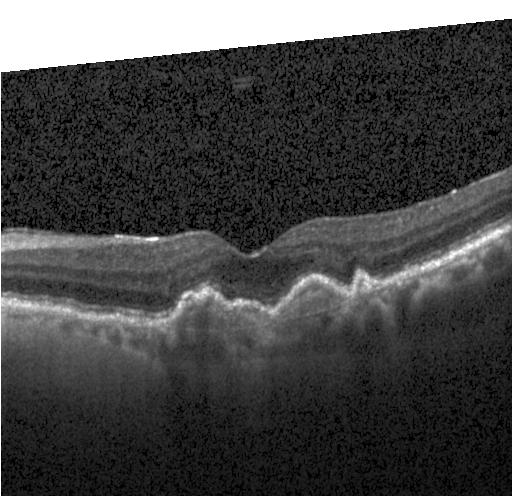
Impression: choroidal neovascularization.